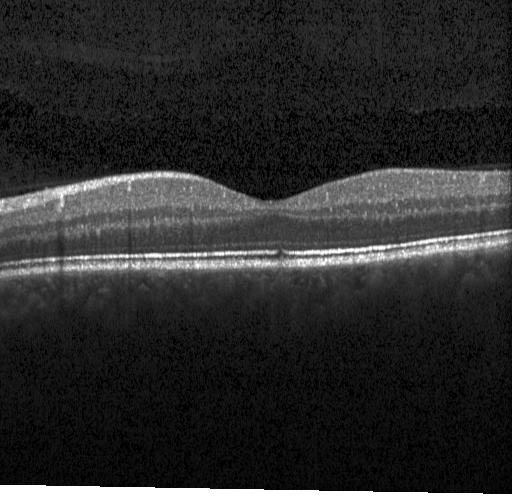

Diagnosis: no choroidal neovascularization, diabetic macular edema, or drusen.